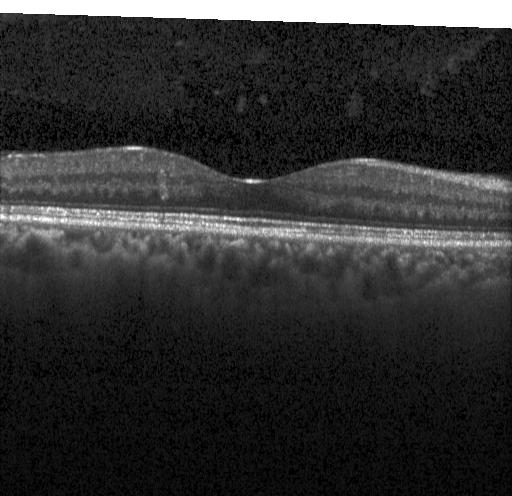 Diagnosis: no CNV, DME, or drusen.